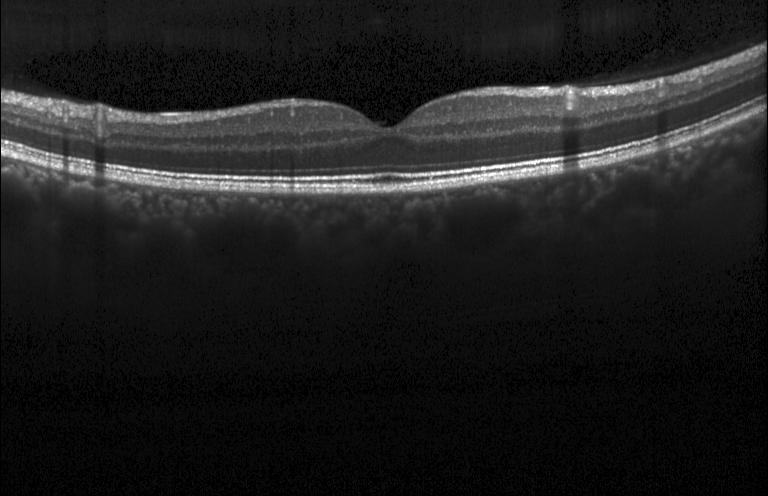 Diagnosis: neither CNV, DME, nor drusen.